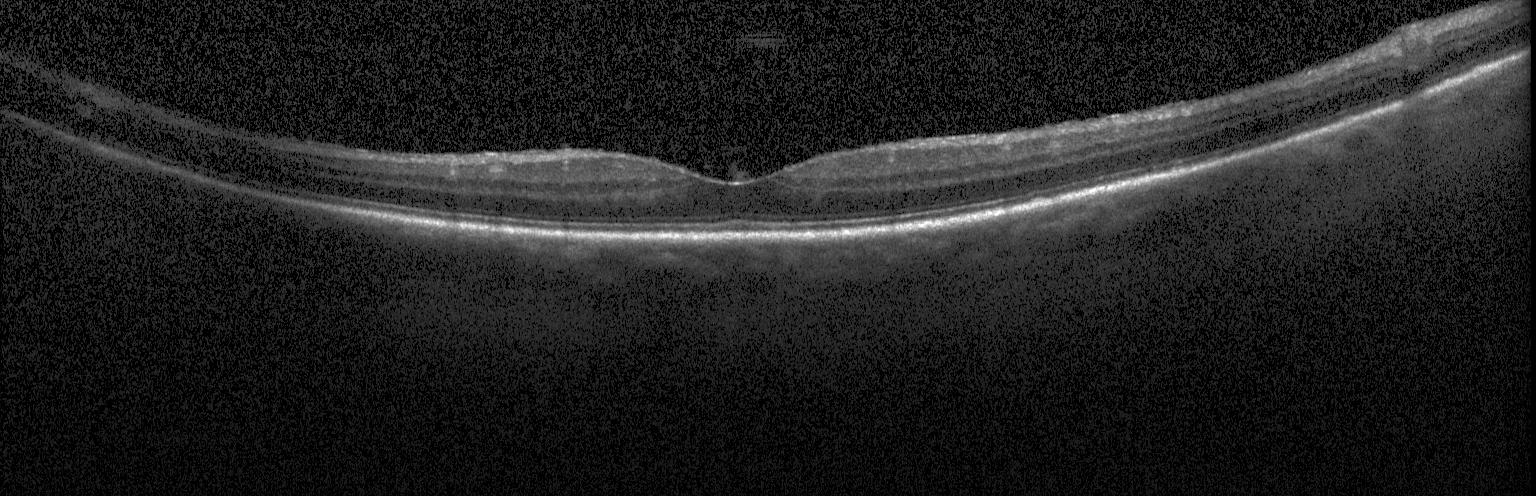 Spectral-domain optical coherence tomography; optical coherence tomography B-scan; macular scan; Heidelberg Spectralis. OCT finding: no choroidal neovascularization, diabetic macular edema, or drusen.